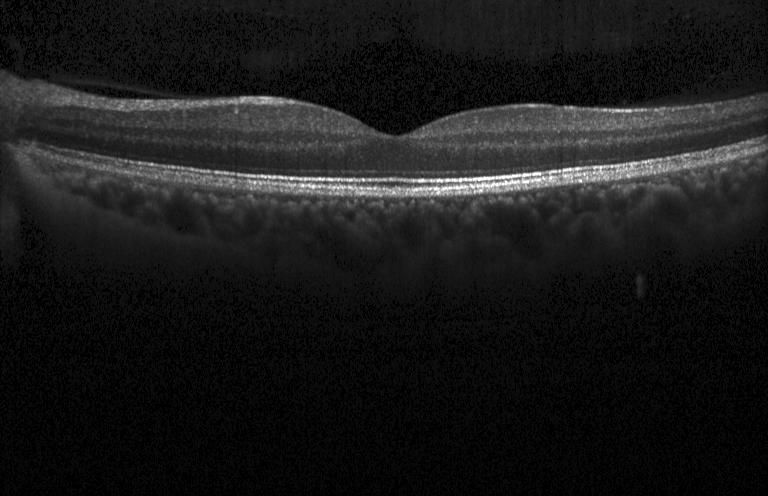

OCT scan showing no choroidal neovascularization, diabetic macular edema, or drusen.